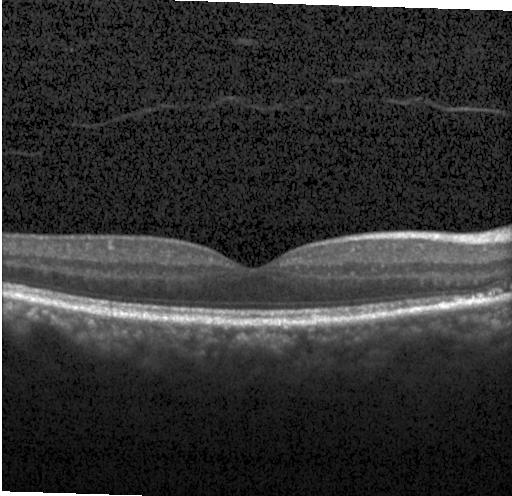
Spectral-domain OCT; Heidelberg Spectralis; OCT line scan.
Impression: no evidence of choroidal neovascularization, diabetic macular edema, or drusen.